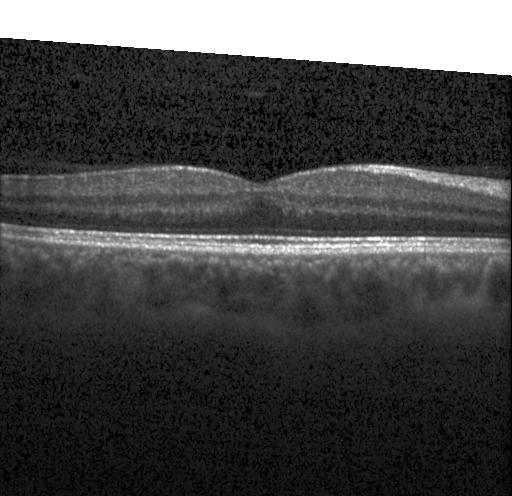 Retinal OCT B-scan
Dx: no choroidal neovascularization, diabetic macular edema, or drusen.